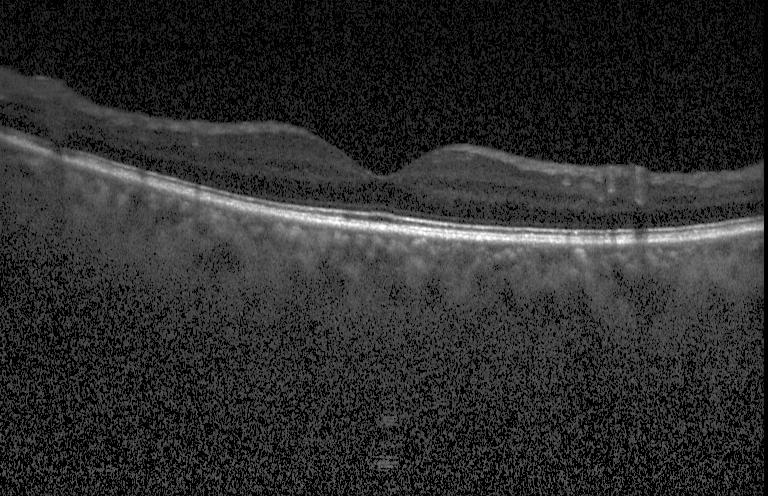 Optical coherence tomography scan. Assessment: no evidence of choroidal neovascularization, diabetic macular edema, or drusen.